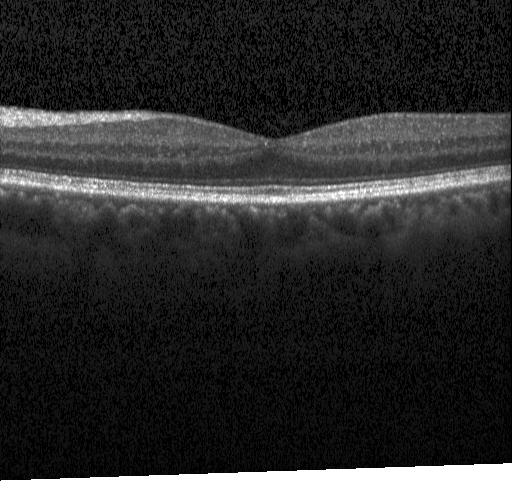
Macular OCT: no evidence of choroidal neovascularization, diabetic macular edema, or drusen.